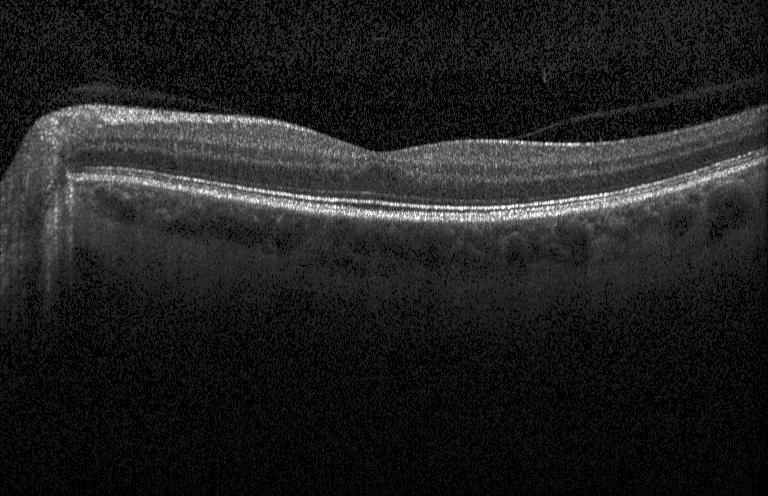

The scan shows no CNV, DME, or drusen.